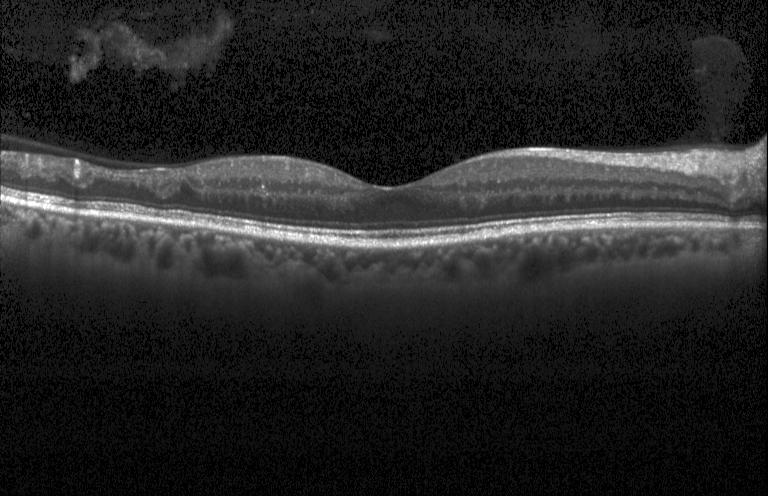

OCT line scan, spectral-domain optical coherence tomography.
OCT finding: neither choroidal neovascularization, diabetic macular edema, nor drusen.